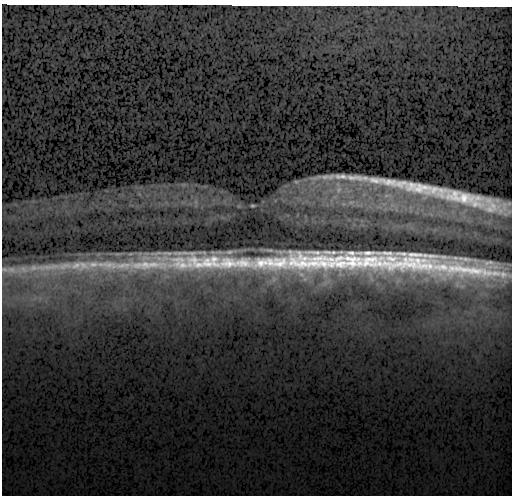

Spectral-domain OCT, centered on the fovea, optical coherence tomography scan, Heidelberg Spectralis. Diagnosis: no CNV, no DME, and no drusen.